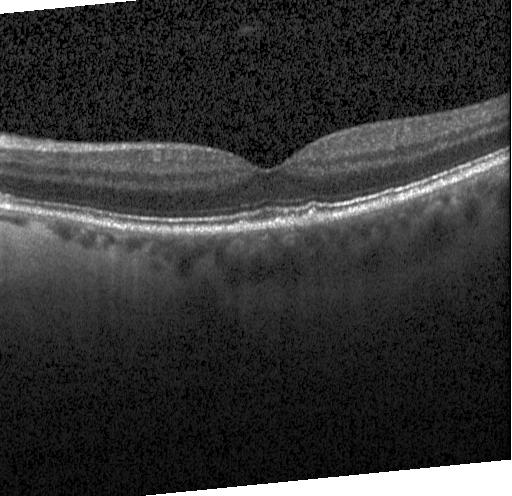

Horizontal scan through the fovea. Spectral-domain OCT. Retinal OCT cross-section — OCT finding: drusen.